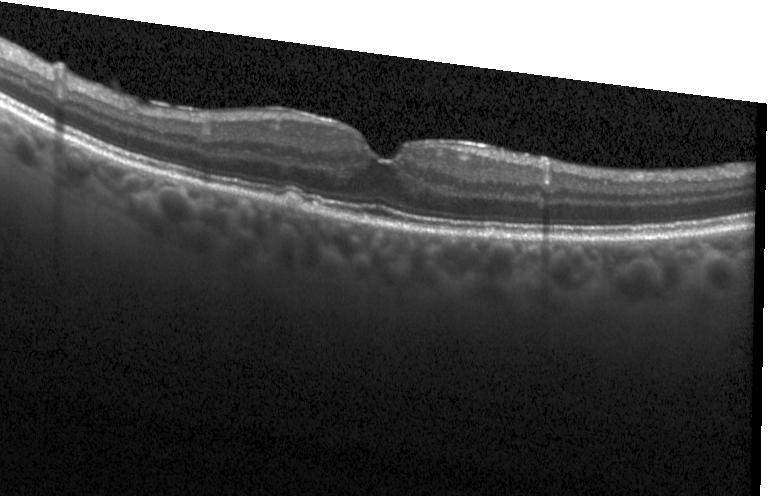 OCT B-scan. Finding: multiple drusen.